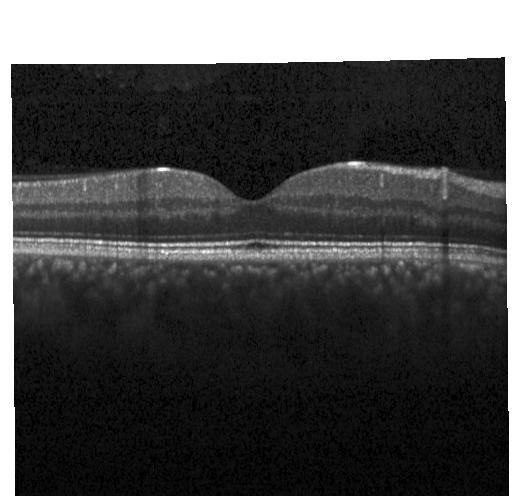
Macular OCT demonstrating no choroidal neovascularization, no diabetic macular edema, and no drusen.